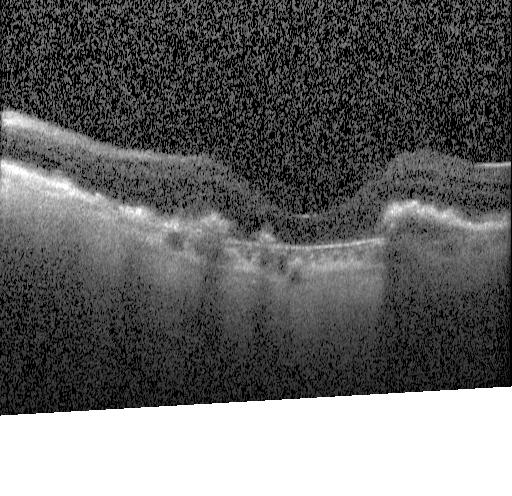

Instrument: Heidelberg Spectralis, optical coherence tomography scan — Impression: a choroidal neovascular membrane.